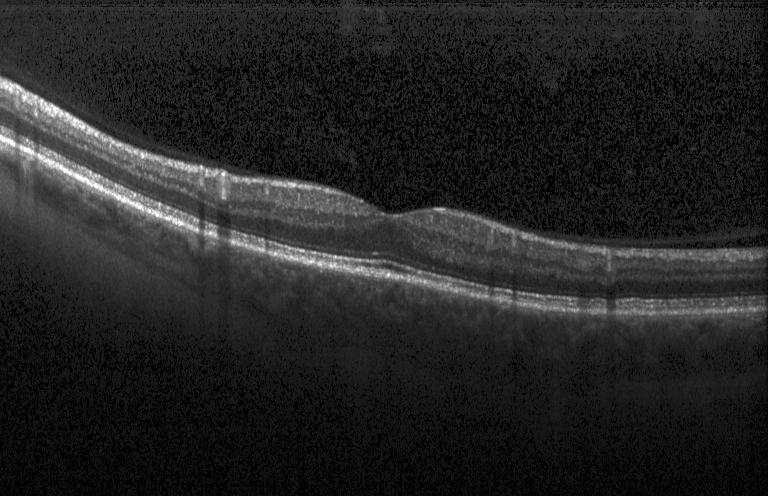

Through the macula, retinal OCT cross-section.
Dx: no CNV, no DME, and no drusen.